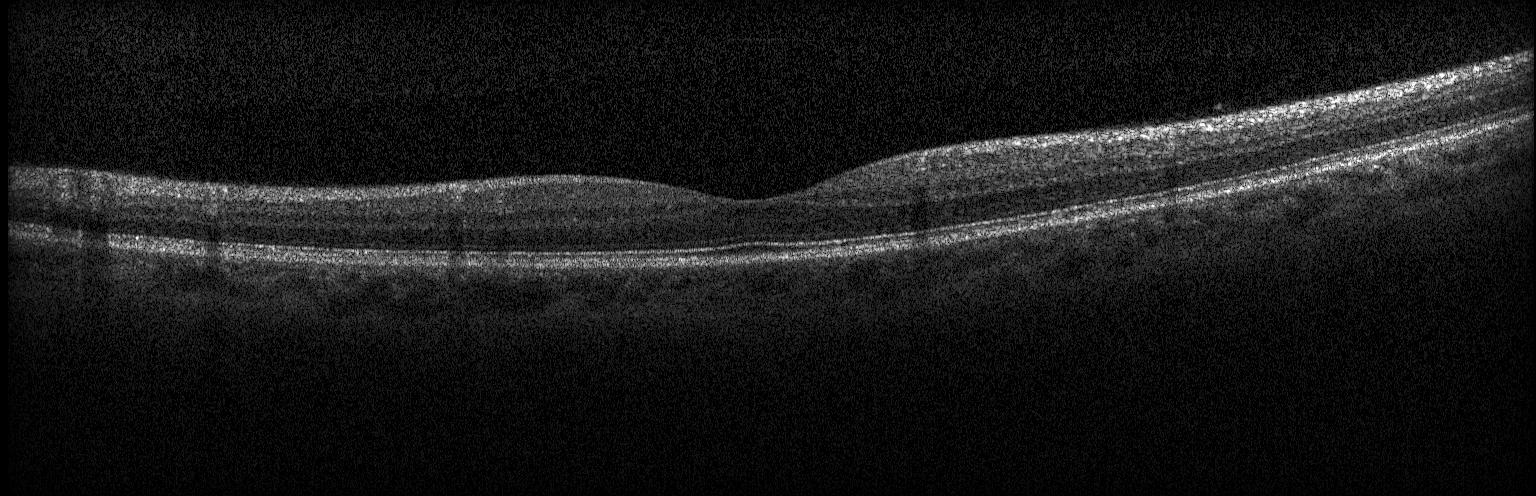

This B-scan demonstrates no choroidal neovascularization, no diabetic macular edema, and no drusen.